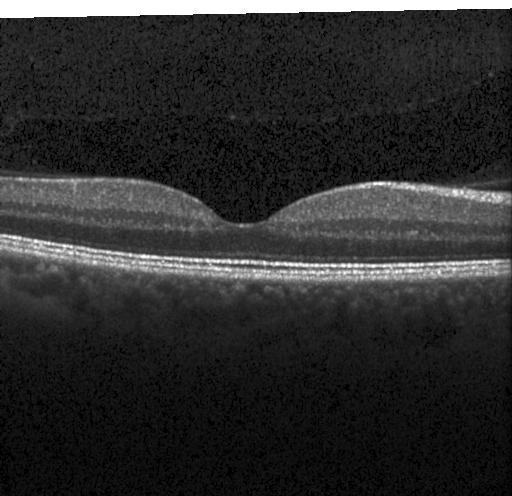
Heidelberg Spectralis OCT system · spectral-domain OCT · through the macula · OCT line scan.
Finding: neither choroidal neovascularization, diabetic macular edema, nor drusen.